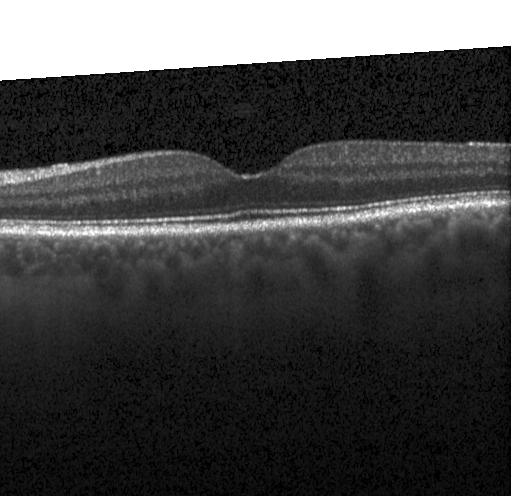
Fovea-centered, acquired on a Heidelberg Spectralis, SD-OCT, optical coherence tomography B-scan — The scan shows no evidence of CNV, DME, or drusen.